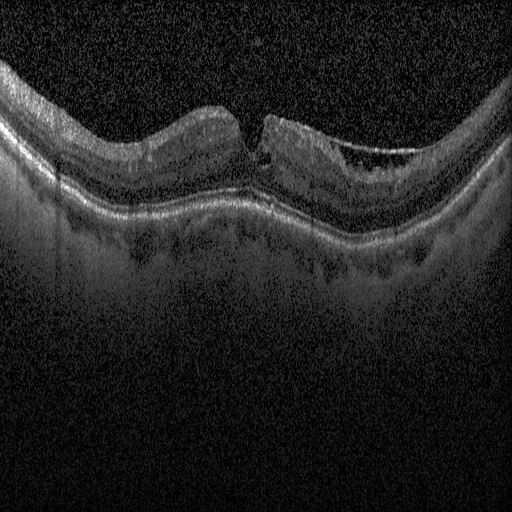 Optical coherence tomography scan. Diagnosis: diabetic macular edema (DME).